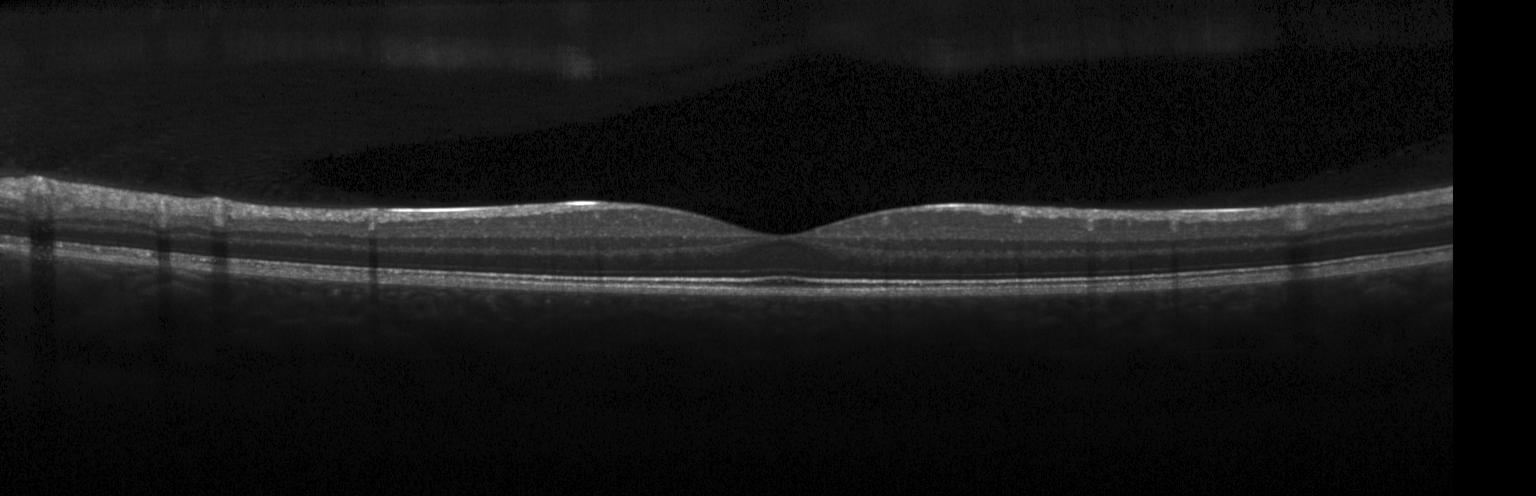 Through the macula; spectral-domain optical coherence tomography; optical coherence tomography scan; Heidelberg Spectralis OCT system
Impression: no choroidal neovascularization, diabetic macular edema, or drusen.